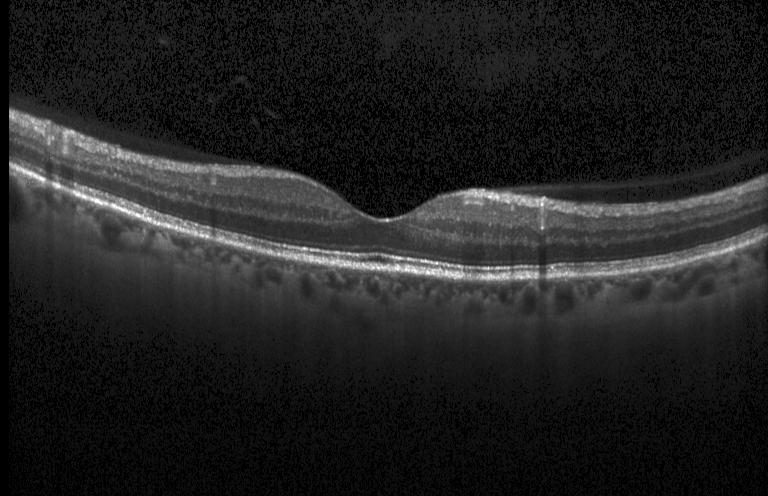

OCT finding: no choroidal neovascularization, diabetic macular edema, or drusen.